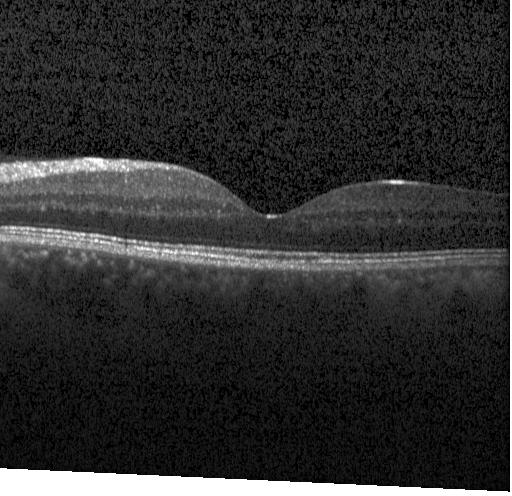 Retinal OCT cross-section — Diagnosis: neither CNV, DME, nor drusen.